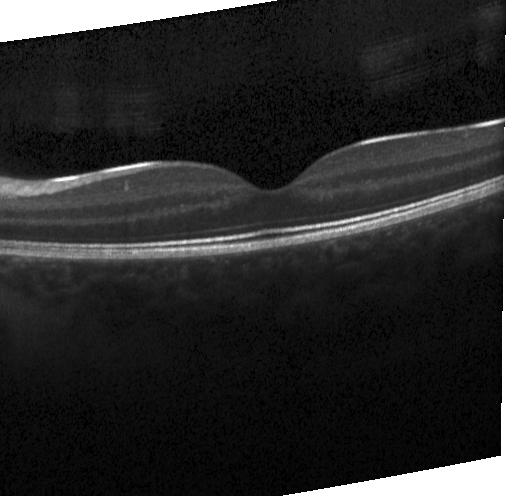

Spectral-domain optical coherence tomography. Heidelberg Spectralis OCT system. Optical coherence tomography scan. Horizontal scan through the fovea
Diagnosis: neither choroidal neovascularization, diabetic macular edema, nor drusen.